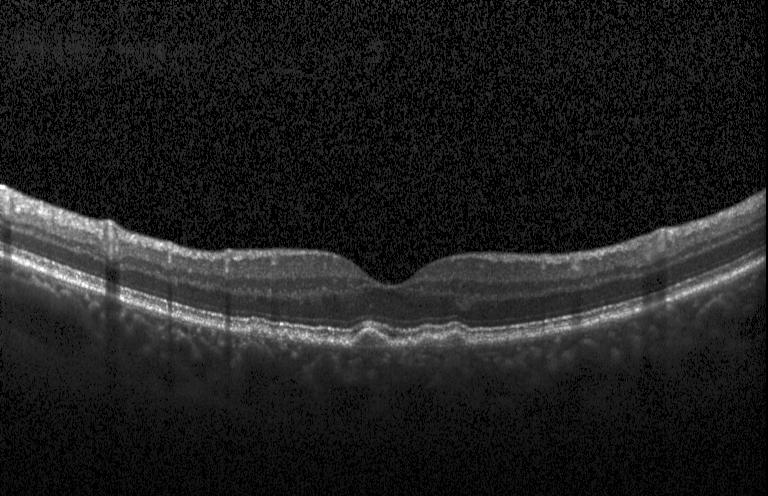 Horizontal scan through the fovea, OCT B-scan, SD-OCT
Dx: sub-RPE drusenoid deposits.